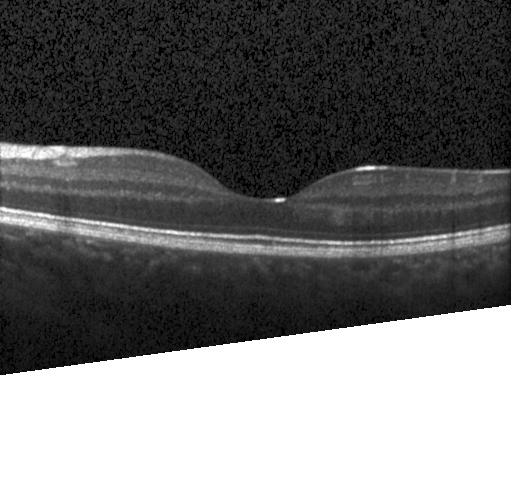
Optical coherence tomography B-scan.
Assessment: no CNV, DME, or drusen.